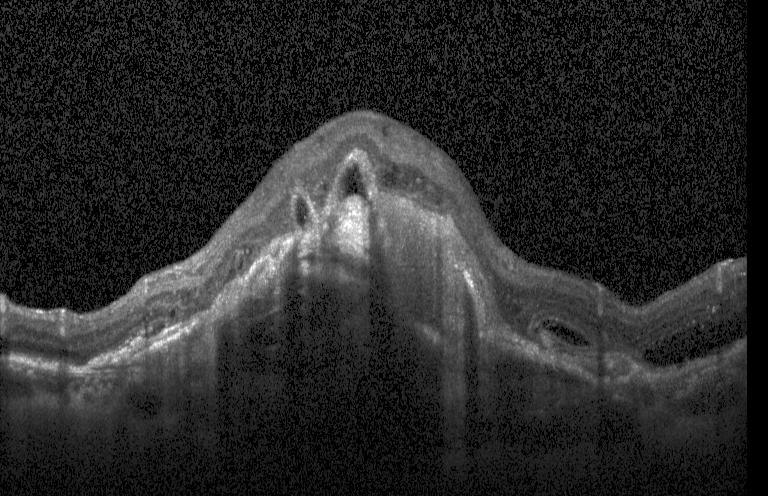

Optical coherence tomography B-scan — Impression: choroidal neovascularization.